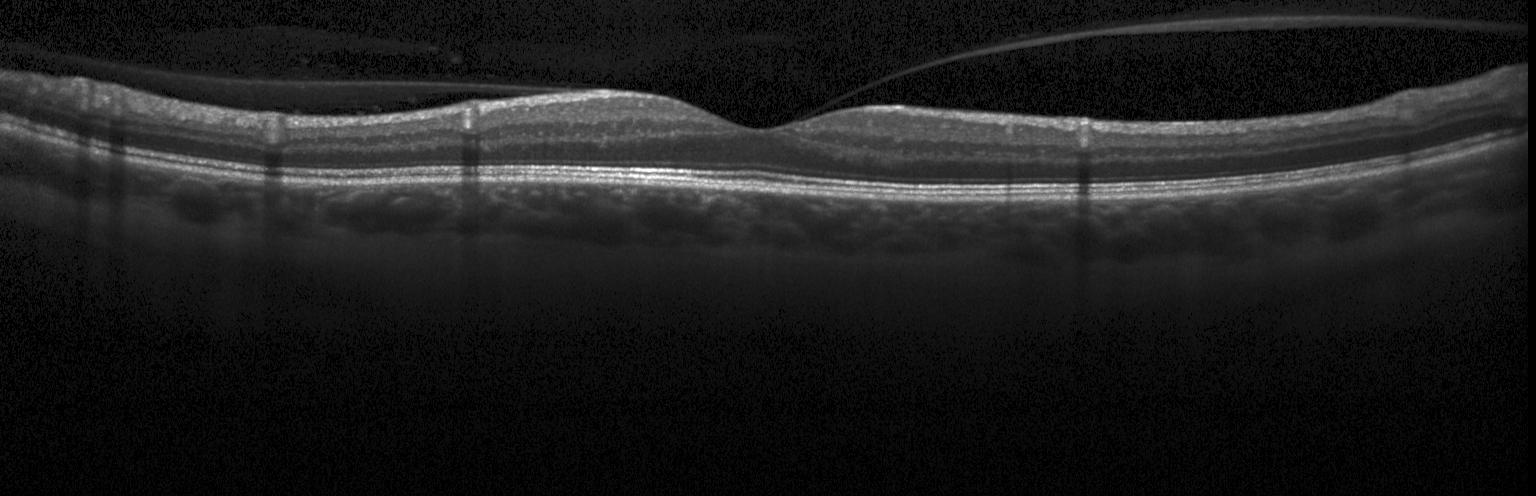

Optical coherence tomography B-scan, fovea-centered, instrument: Heidelberg Spectralis — The scan shows no choroidal neovascularization, no diabetic macular edema, and no drusen.